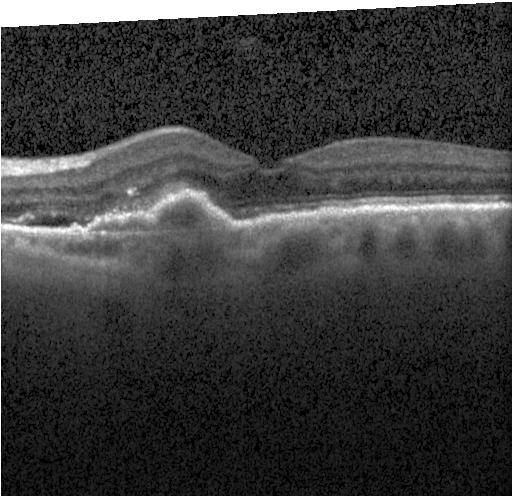
SD-OCT. Horizontal scan through the fovea. Acquired on a Heidelberg Spectralis. Optical coherence tomography scan. The scan shows choroidal neovascularization (CNV).